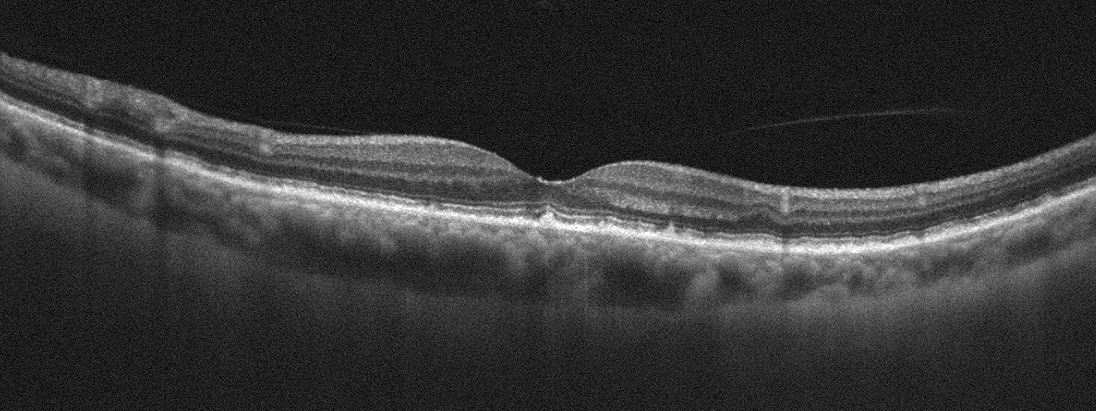
Assessment: AMD.